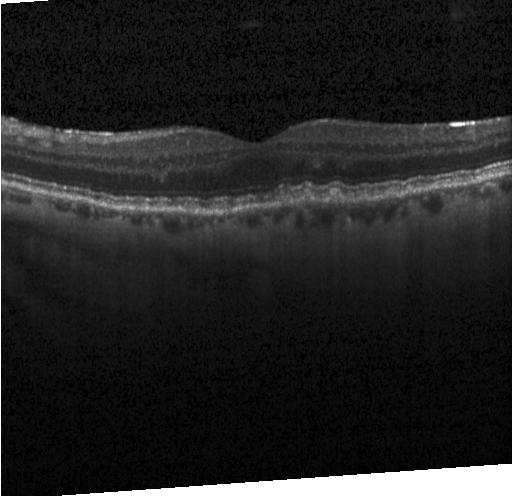
OCT line scan. OCT finding: multiple drusen.